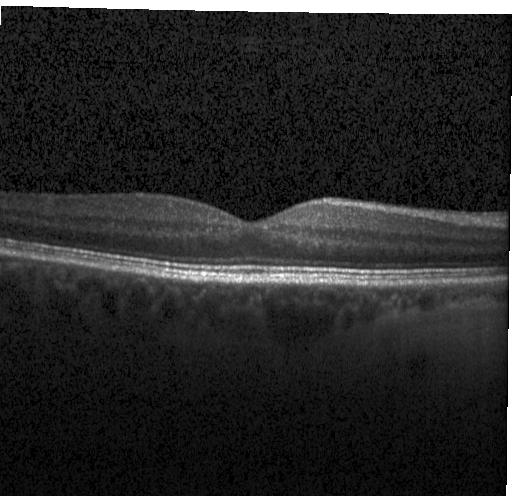

Instrument: Heidelberg Spectralis. Through the macula. Spectral-domain OCT. Optical coherence tomography scan.
Assessment: no choroidal neovascularization, no diabetic macular edema, and no drusen.